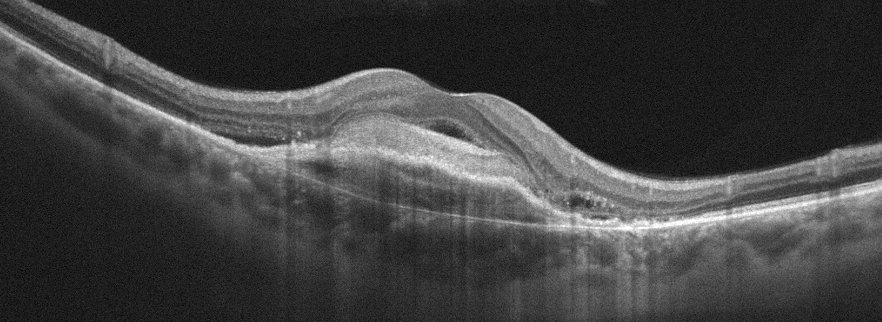
Right eye; retinal OCT cross-section — Finding: age-related macular degeneration.